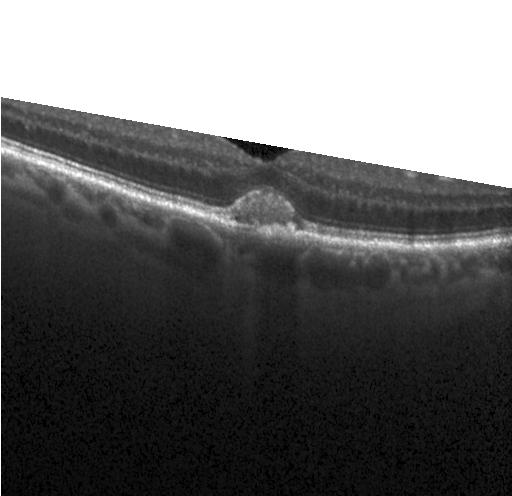
The scan shows CNV.